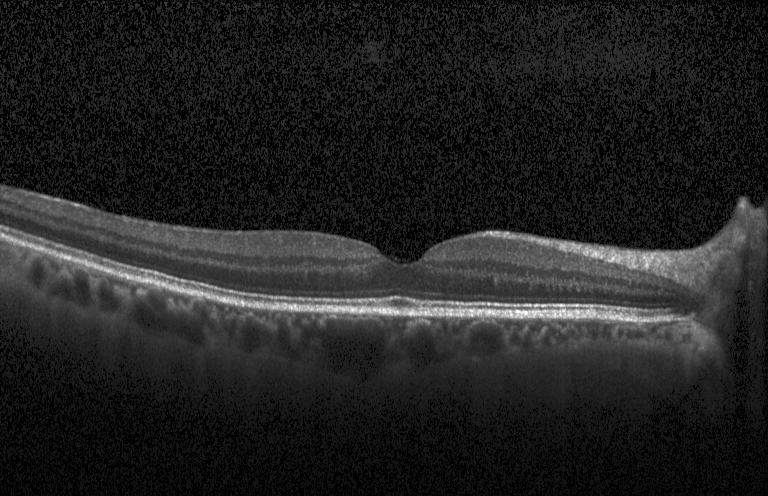 OCT B-scan. SD-OCT — Finding: no evidence of choroidal neovascularization, diabetic macular edema, or drusen.